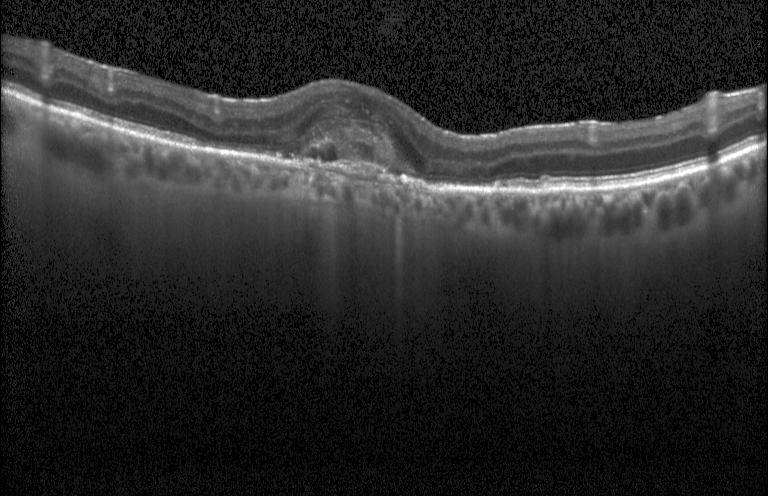

Retinal OCT cross-section — Diagnosis: choroidal neovascularization (CNV).